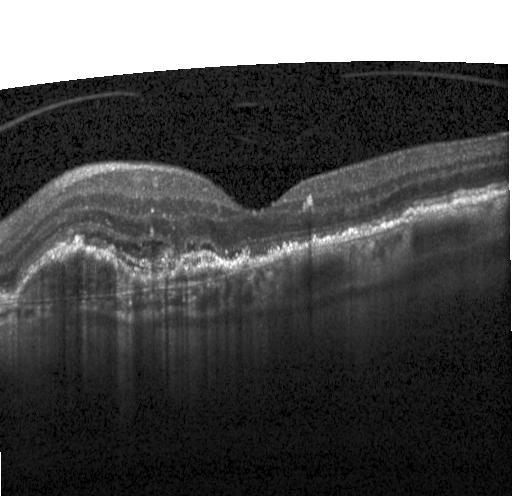

The scan shows choroidal neovascularization (CNV).